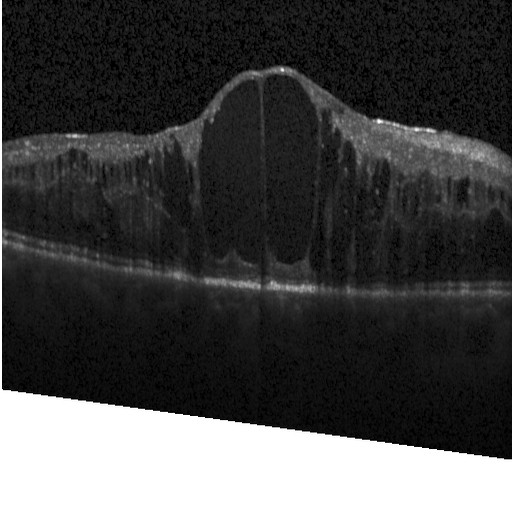

DME.